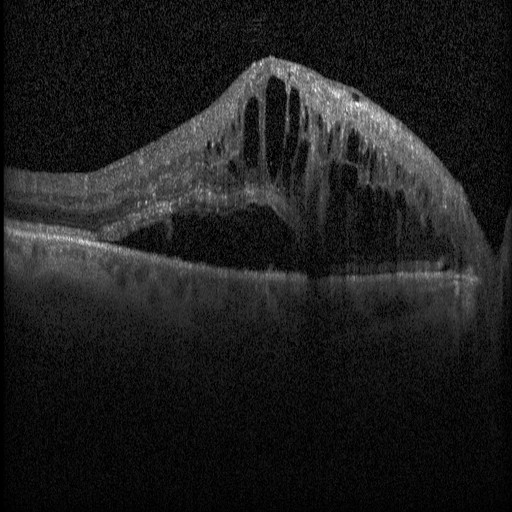 Dx: diabetic macular edema (DME).